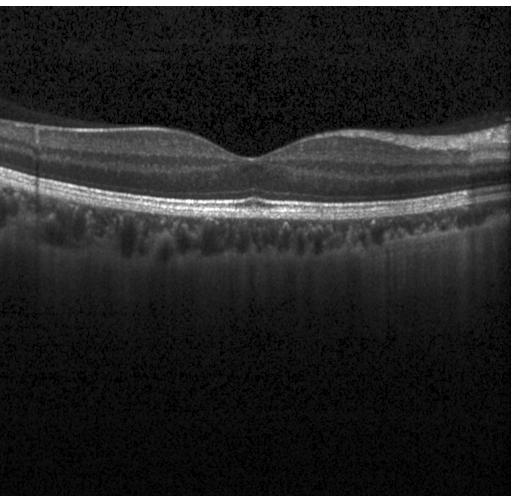
OCT line scan — Assessment: neither choroidal neovascularization, diabetic macular edema, nor drusen.